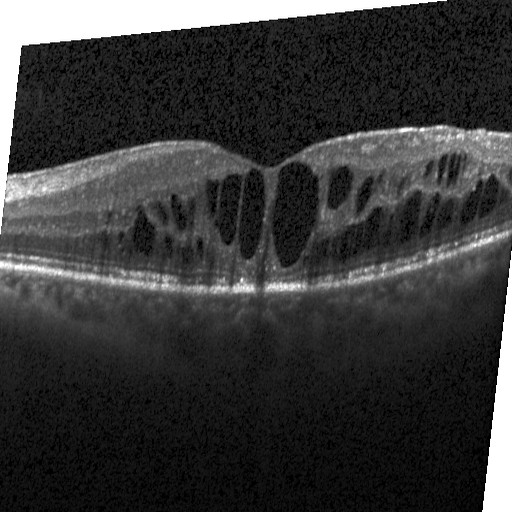 Centered on the fovea. OCT line scan. Spectral-domain OCT. Heidelberg Spectralis — Impression: DME.